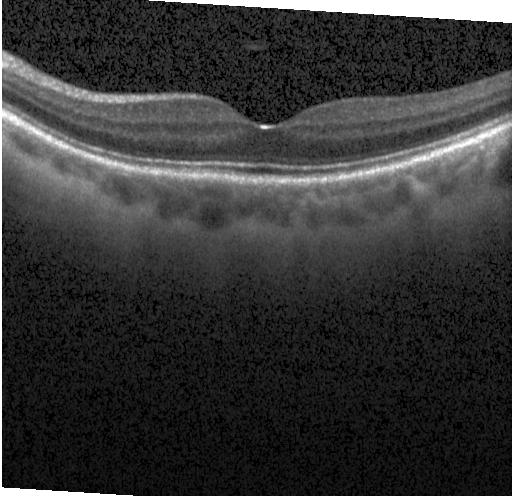 Through the macula. Retinal OCT B-scan. Assessment: no evidence of choroidal neovascularization, diabetic macular edema, or drusen.